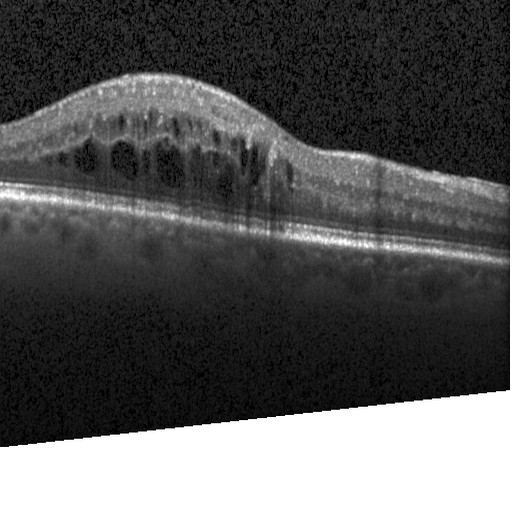
This B-scan demonstrates diabetic macular edema.